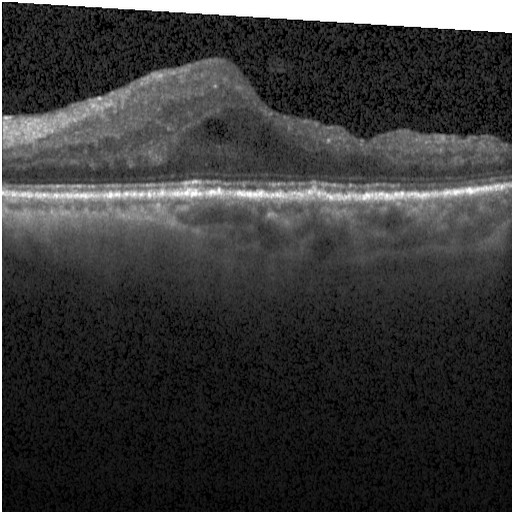

Instrument: Heidelberg Spectralis; optical coherence tomography scan.
Impression: diabetic macular edema.